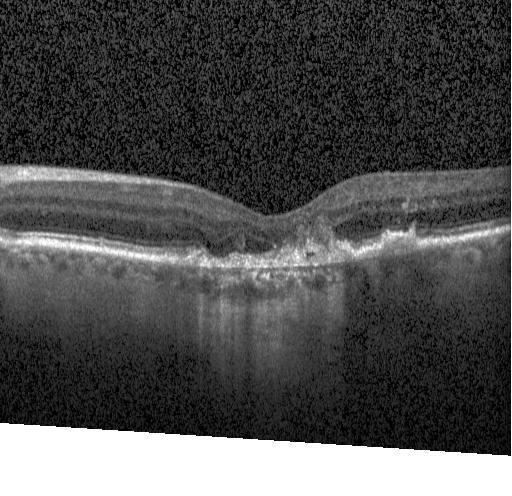
Heidelberg Spectralis OCT system · spectral-domain OCT · horizontal scan through the fovea · optical coherence tomography B-scan. Finding: choroidal neovascularization.